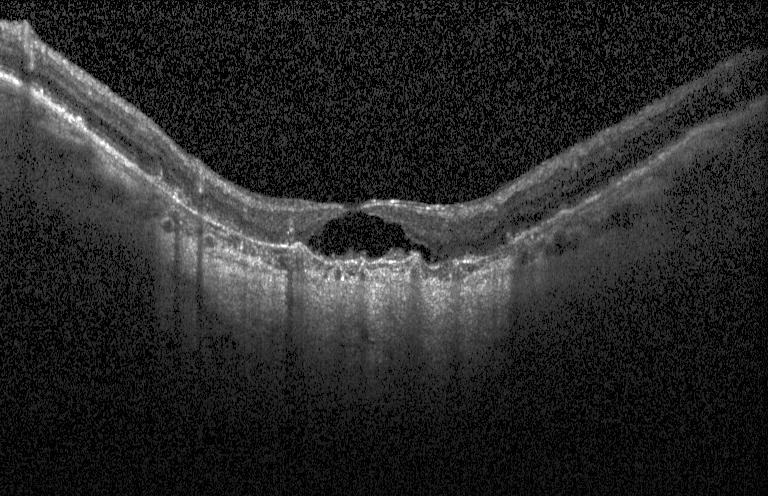 Retinal OCT cross-section.
Finding: choroidal neovascularization.